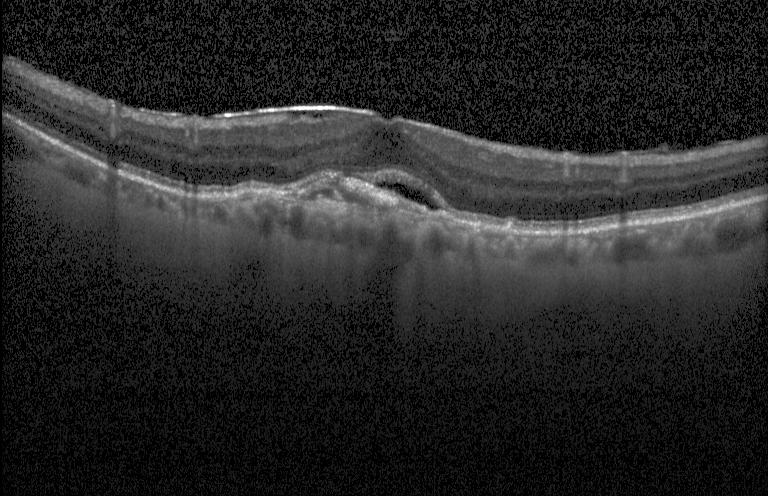
Macular scan; retinal OCT cross-section; spectral-domain OCT — Choroidal neovascularization (CNV).